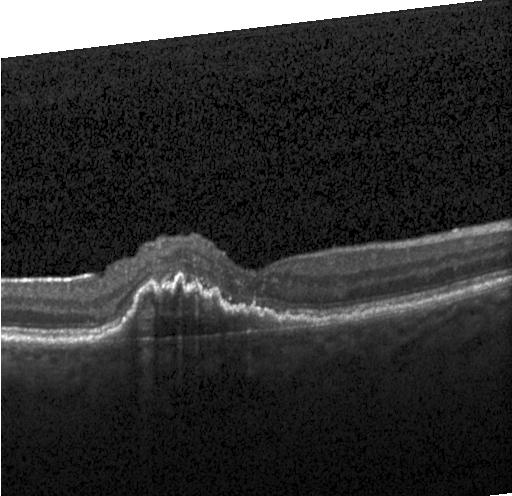 Retinal OCT cross-section showing a choroidal neovascular membrane.